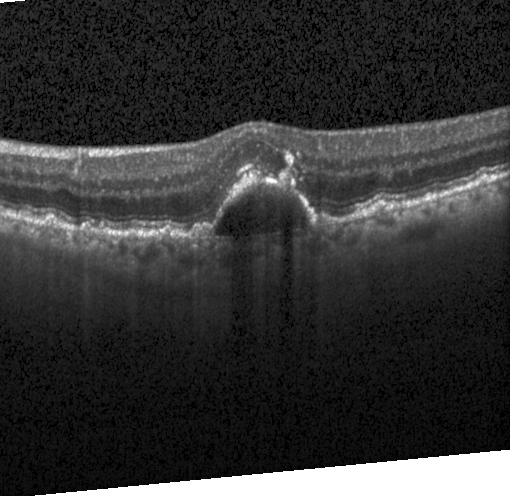

Optical coherence tomography B-scan
Impression: CNV.